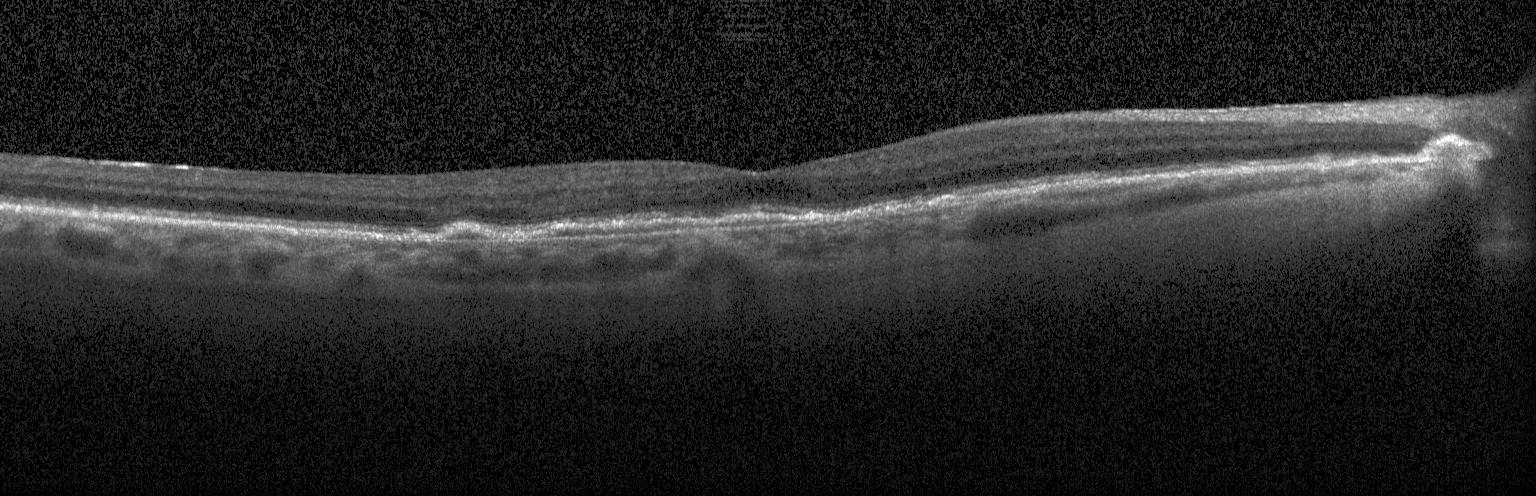
CNV.